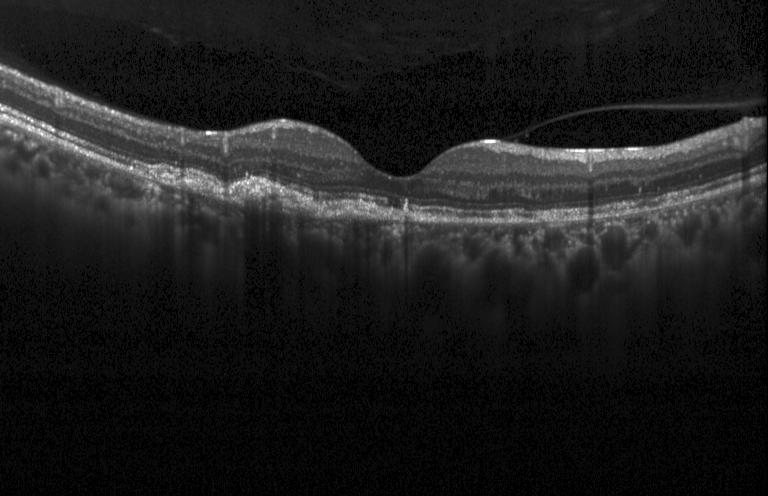 Fovea-centered, retinal OCT B-scan, acquired on a Heidelberg Spectralis, spectral-domain OCT.
OCT finding: choroidal neovascularization (CNV).